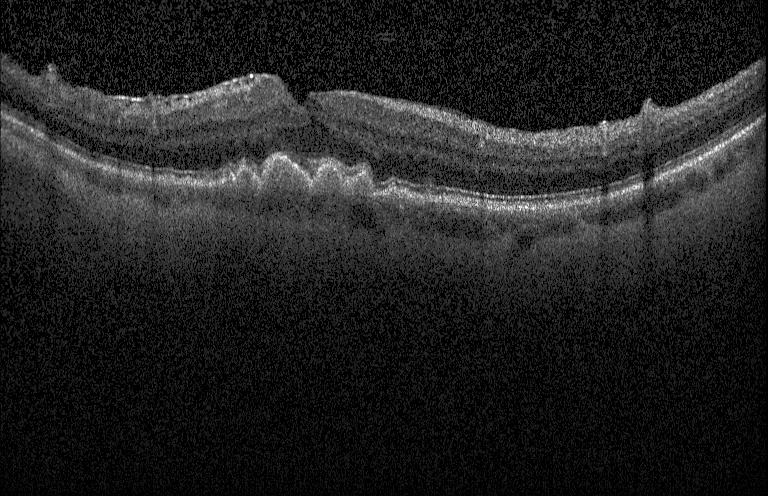
OCT B-scan. The scan shows multiple drusen.